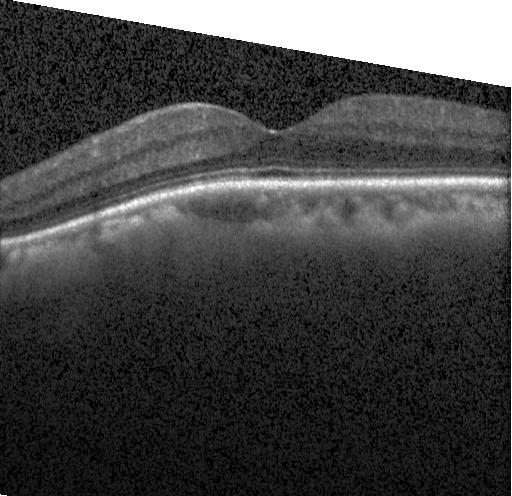
Retinal OCT B-scan.
Diagnosis: neither choroidal neovascularization, diabetic macular edema, nor drusen.